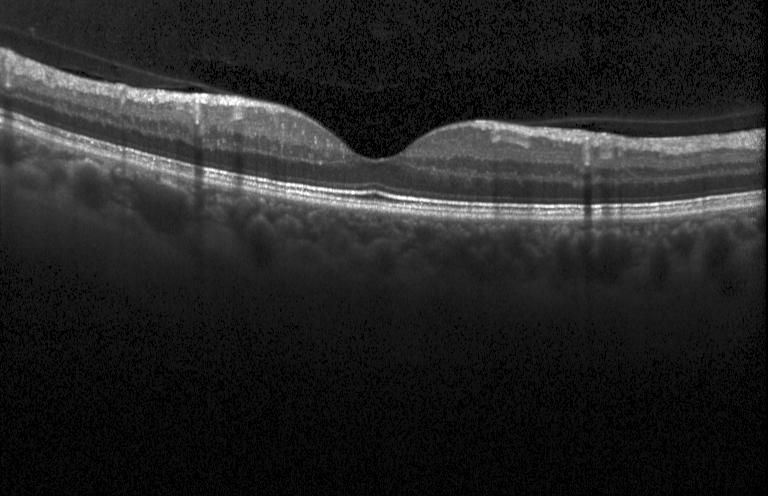

Spectral-domain OCT. Macular scan. Retinal OCT cross-section. Heidelberg Spectralis.
Finding: neither choroidal neovascularization, diabetic macular edema, nor drusen.